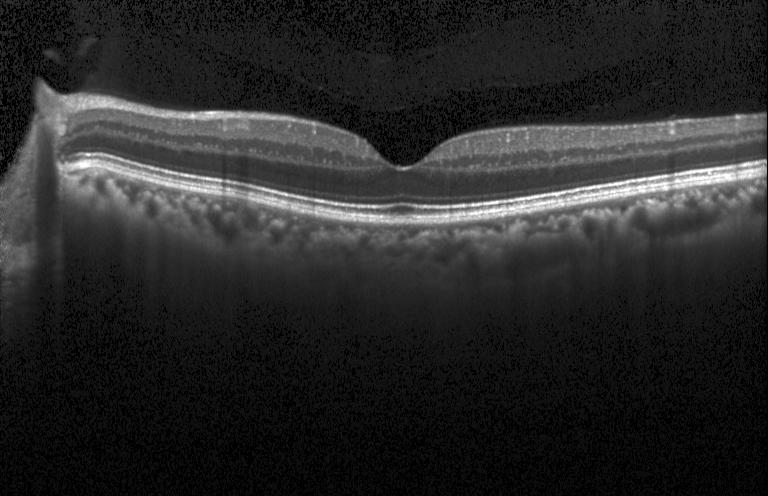 Diagnosis: no evidence of CNV, DME, or drusen.